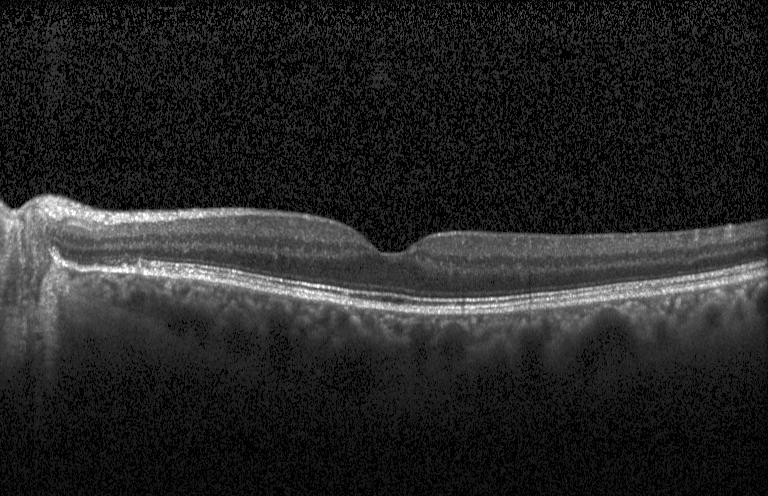

Spectral-domain OCT. Retinal OCT cross-section.
Macular OCT: no choroidal neovascularization, no diabetic macular edema, and no drusen.